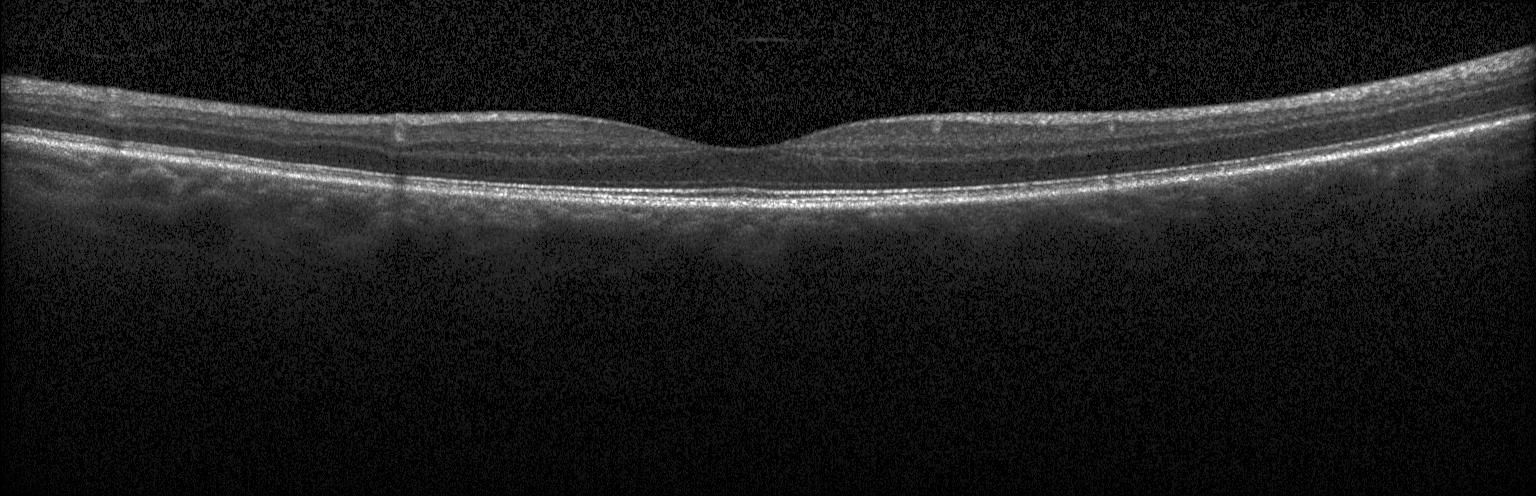

Optical coherence tomography B-scan.
Impression: no evidence of choroidal neovascularization, diabetic macular edema, or drusen.